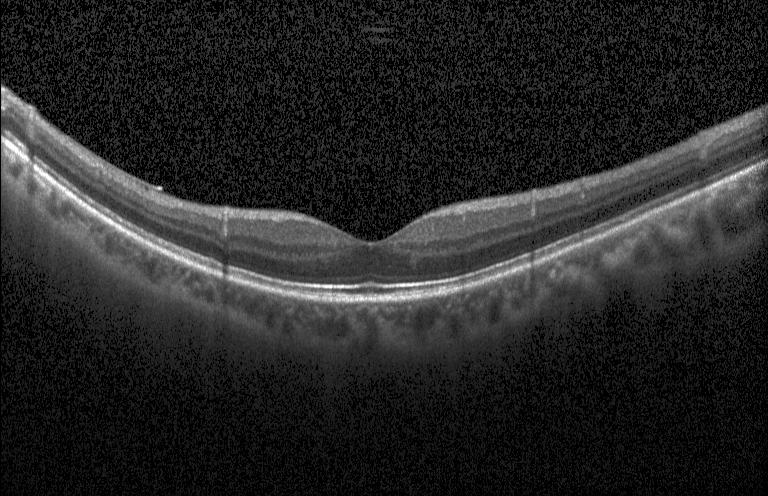 No choroidal neovascularization, no diabetic macular edema, and no drusen.